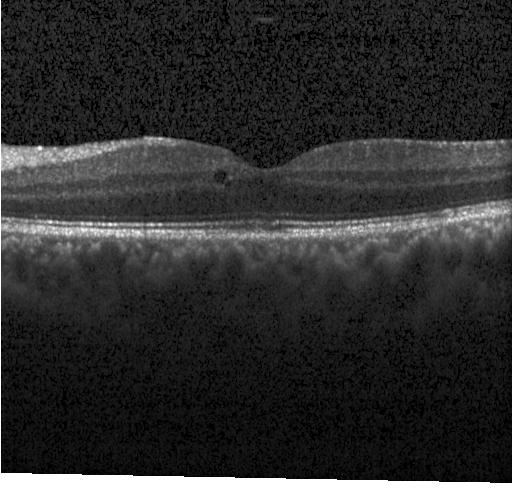

Heidelberg Spectralis OCT system, SD-OCT, fovea-centered, retinal OCT B-scan — Finding: diabetic macular edema.